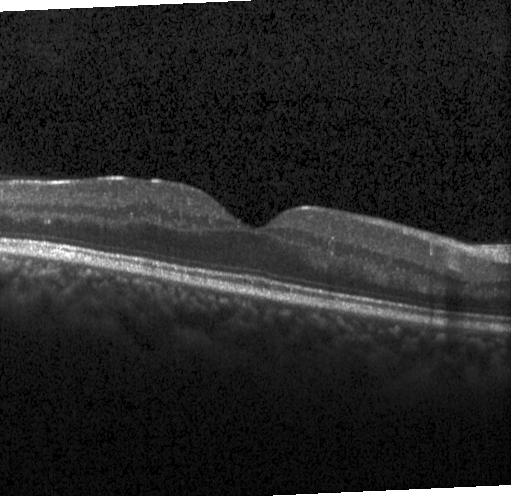
Centered on the fovea; retinal OCT B-scan; acquired on a Heidelberg Spectralis; SD-OCT.
Finding: no choroidal neovascularization, no diabetic macular edema, and no drusen.